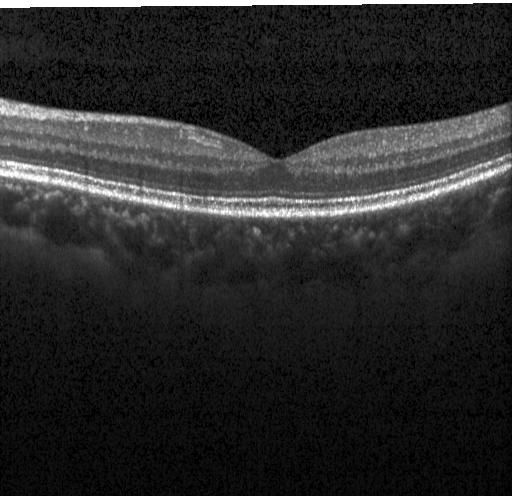

OCT scan showing no CNV, DME, or drusen.